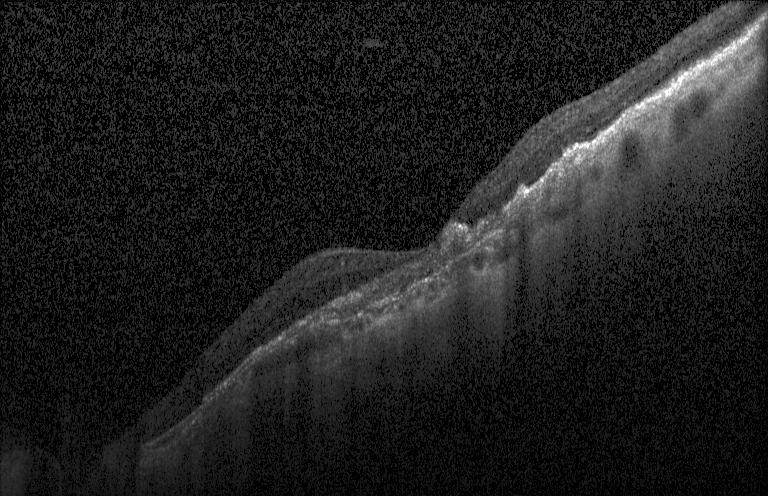

Macular OCT demonstrating choroidal neovascularization.